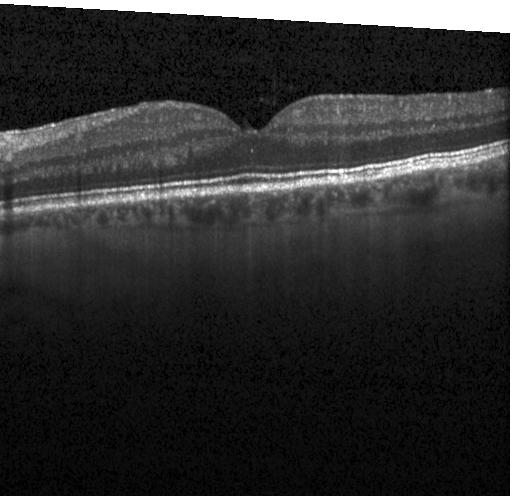

Spectral-domain optical coherence tomography, retinal OCT cross-section, acquired on a Heidelberg Spectralis. Impression: no CNV, no DME, and no drusen.